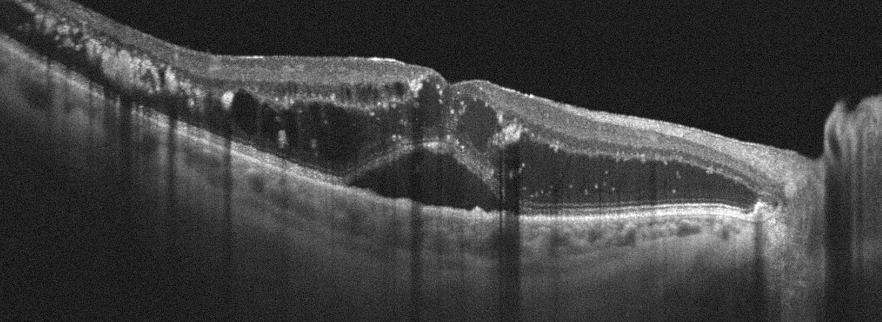

Instrument: Optovue Avanti RTVue XR. OCT B-scan. Through the macula — Impression: retinal vein occlusion.